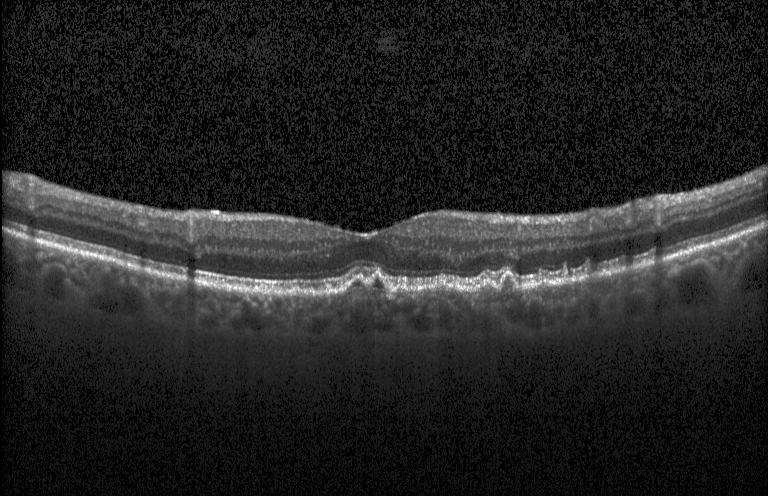
Optical coherence tomography scan; SD-OCT; Heidelberg Spectralis — Finding: multiple drusen.